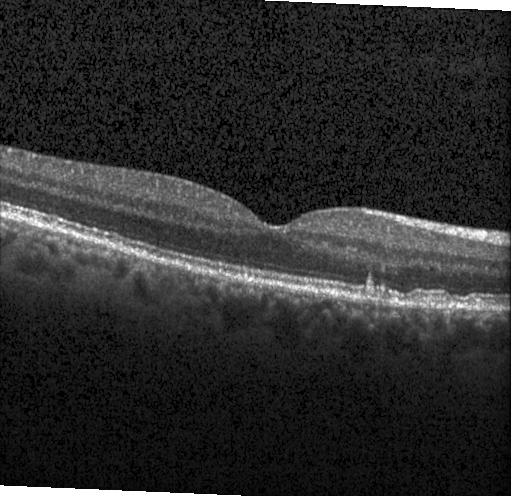
Macular OCT demonstrating drusen.